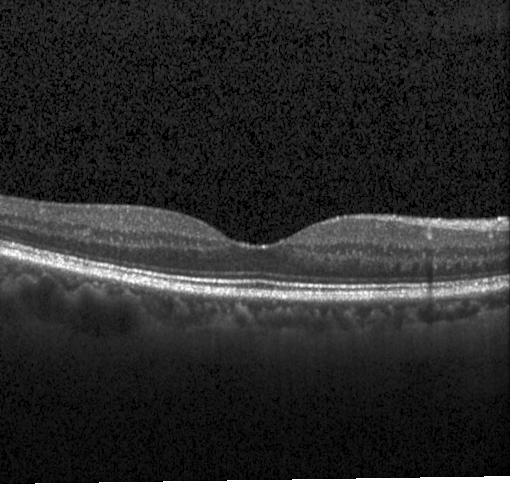
Impression: no evidence of CNV, DME, or drusen.